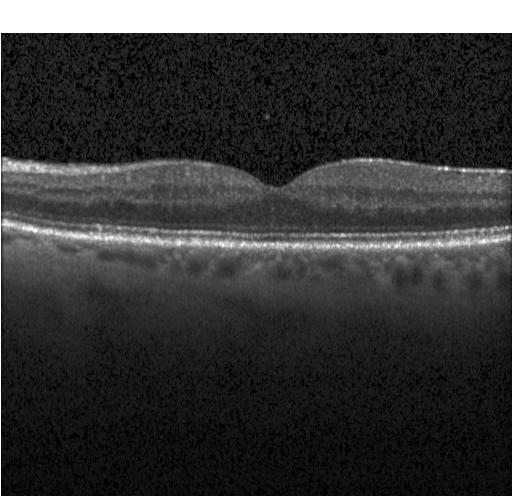 Centered on the fovea; OCT B-scan; acquired on a Heidelberg Spectralis. The scan shows neither CNV, DME, nor drusen.